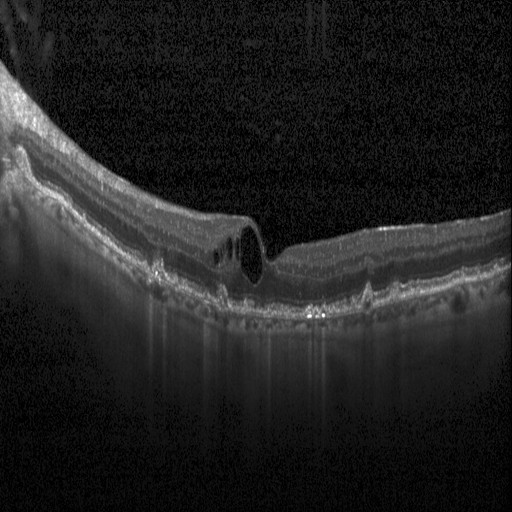 Centered on the fovea; SD-OCT; optical coherence tomography B-scan; instrument: Heidelberg Spectralis. Diagnosis: diabetic macular edema (DME).